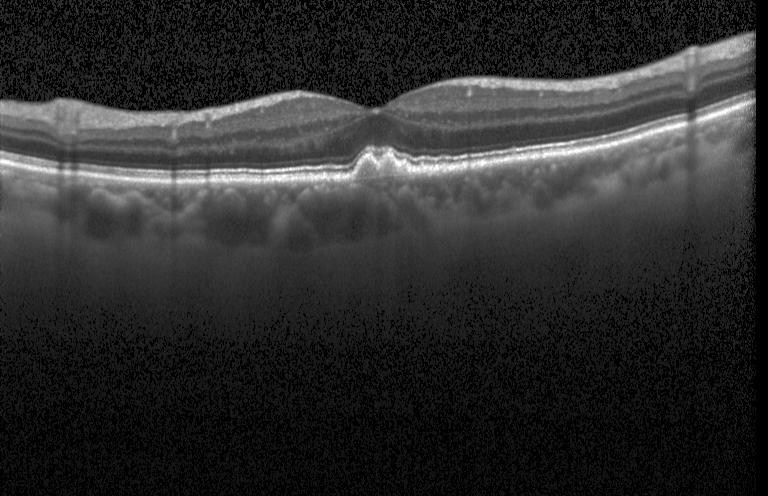 Finding: drusen.